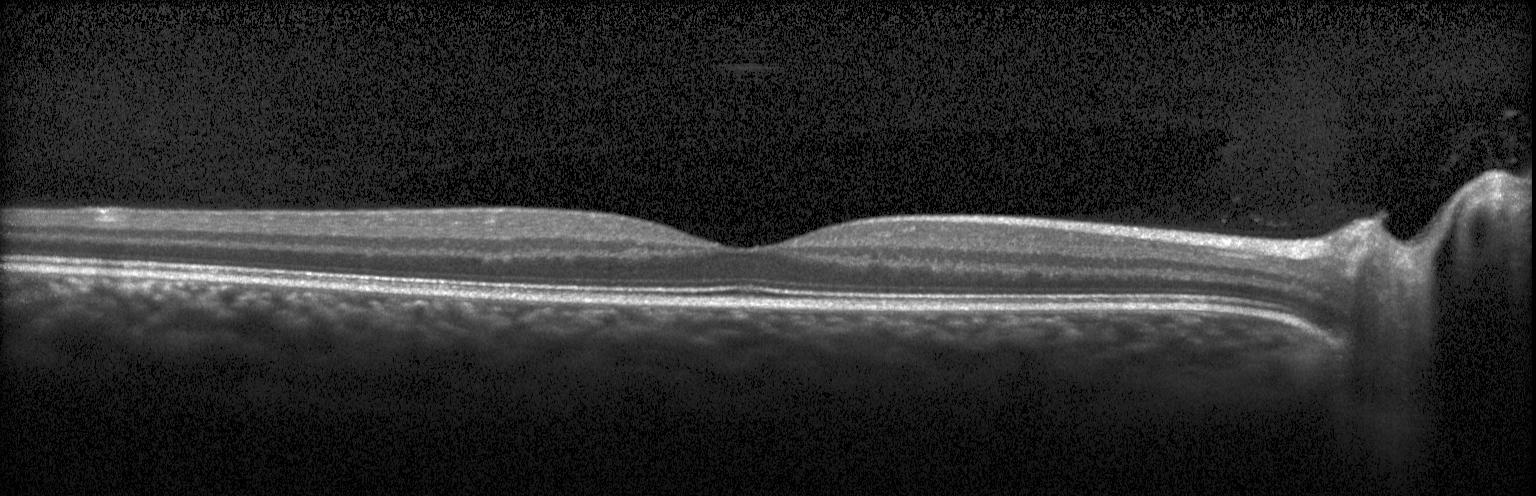 Optical coherence tomography scan; Heidelberg Spectralis OCT system; spectral-domain optical coherence tomography.
This B-scan demonstrates no CNV, DME, or drusen.